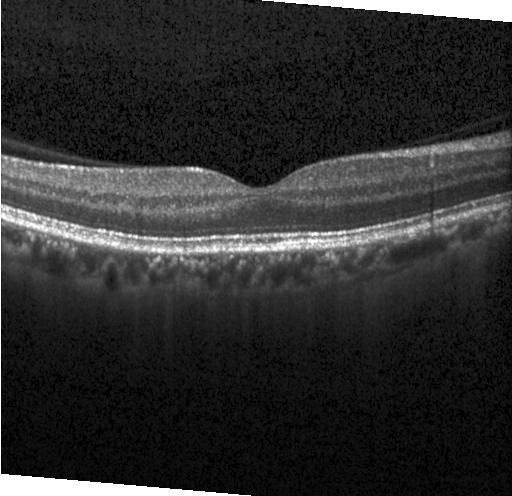 Finding: no evidence of CNV, DME, or drusen.